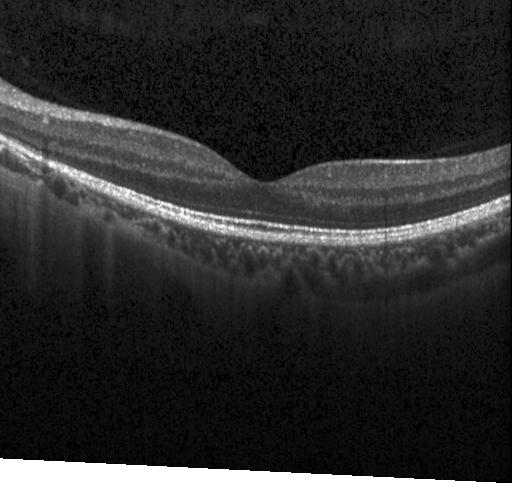 Centered on the fovea, Heidelberg Spectralis OCT system, OCT B-scan, spectral-domain OCT — Finding: no CNV, no DME, and no drusen.